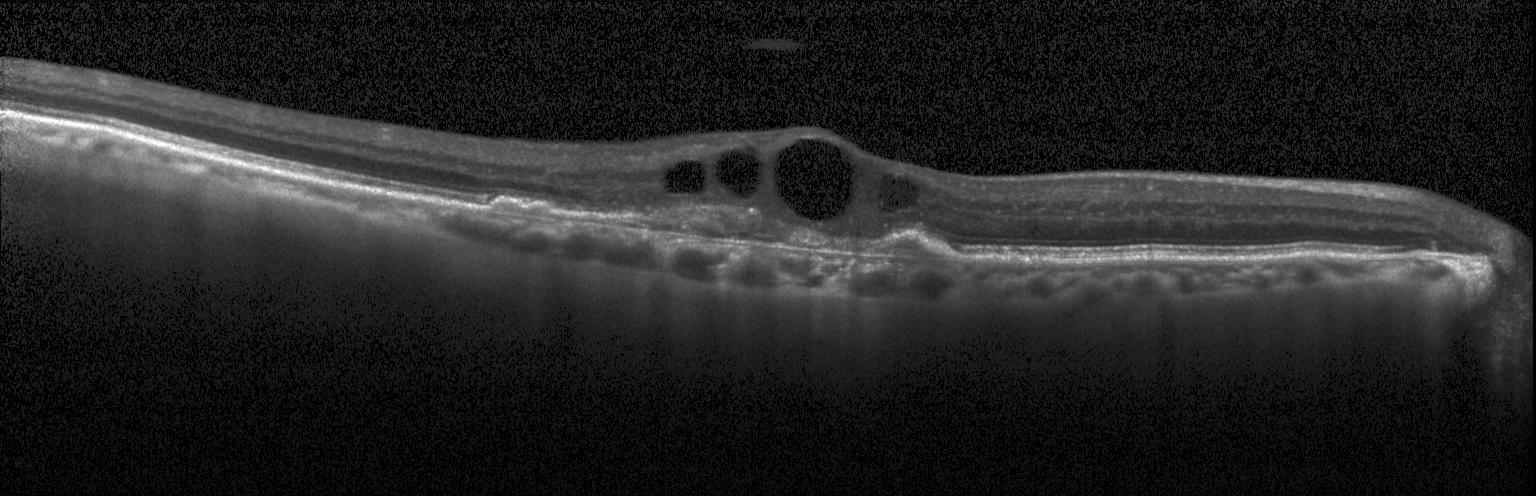
Macular OCT demonstrating a choroidal neovascular membrane.